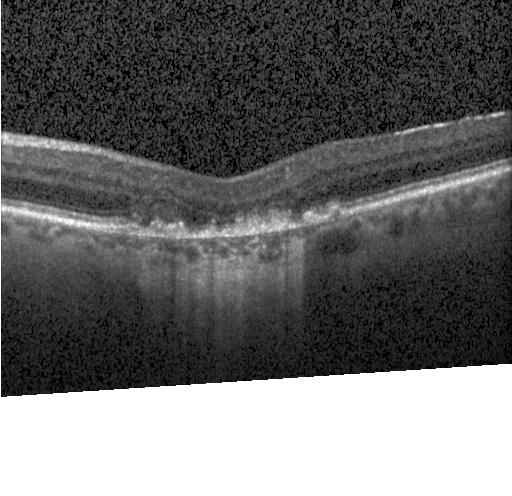 Diagnosis: choroidal neovascularization (CNV).